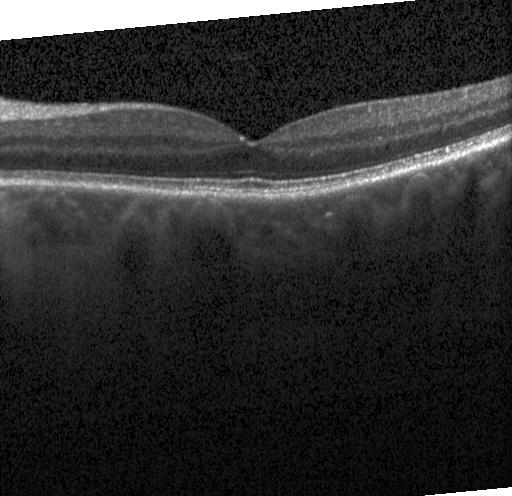
OCT B-scan — Macular OCT: neither choroidal neovascularization, diabetic macular edema, nor drusen.